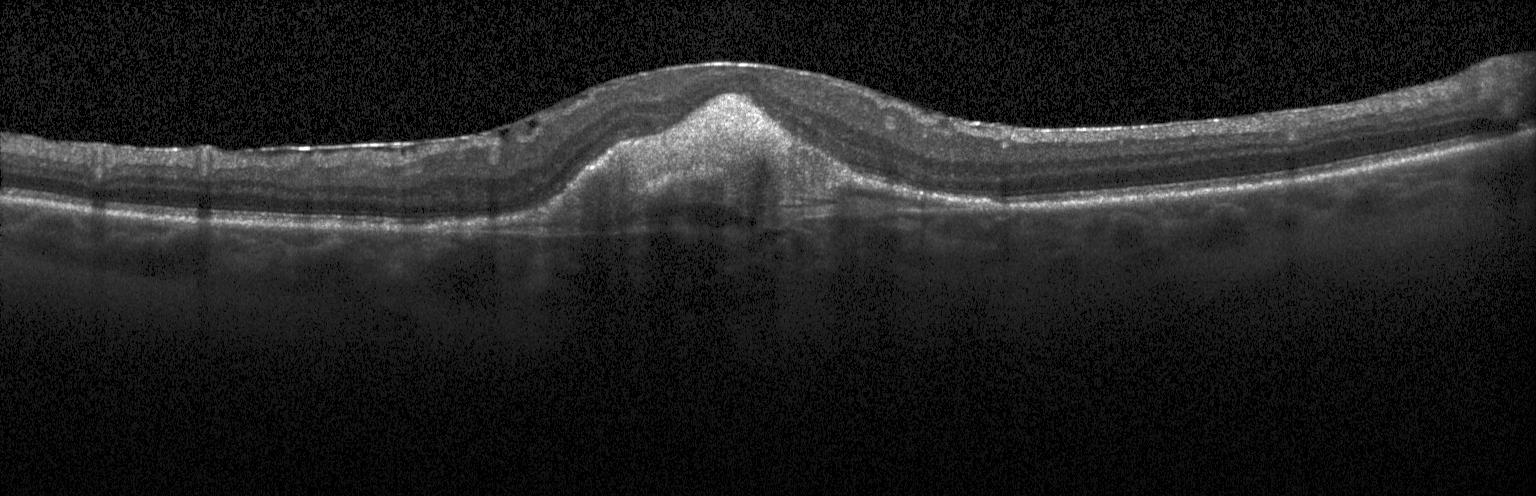 OCT line scan — Choroidal neovascularization.